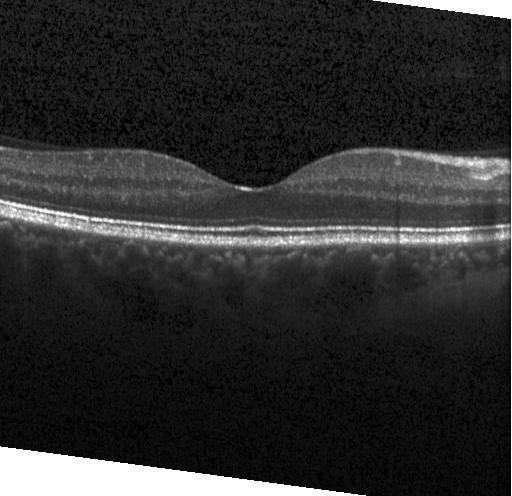

Spectral-domain optical coherence tomography. OCT line scan. Through the macula
This B-scan demonstrates no evidence of choroidal neovascularization, diabetic macular edema, or drusen.